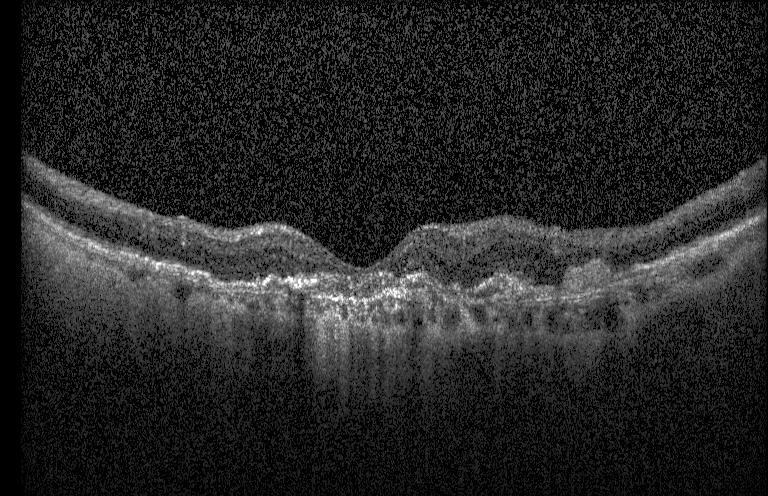 Horizontal scan through the fovea, Heidelberg Spectralis OCT system, OCT B-scan, spectral-domain OCT. Dx: choroidal neovascularization.